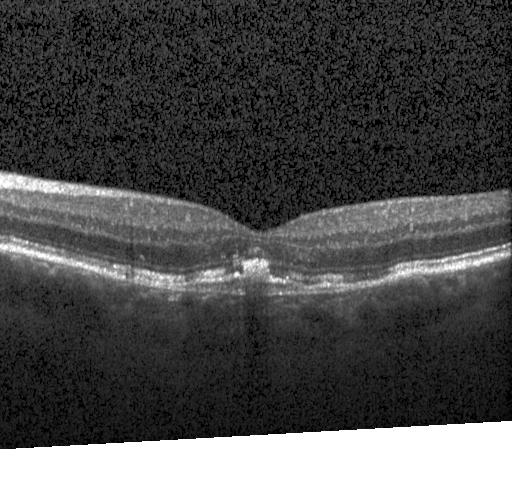

Dx: a choroidal neovascular membrane.